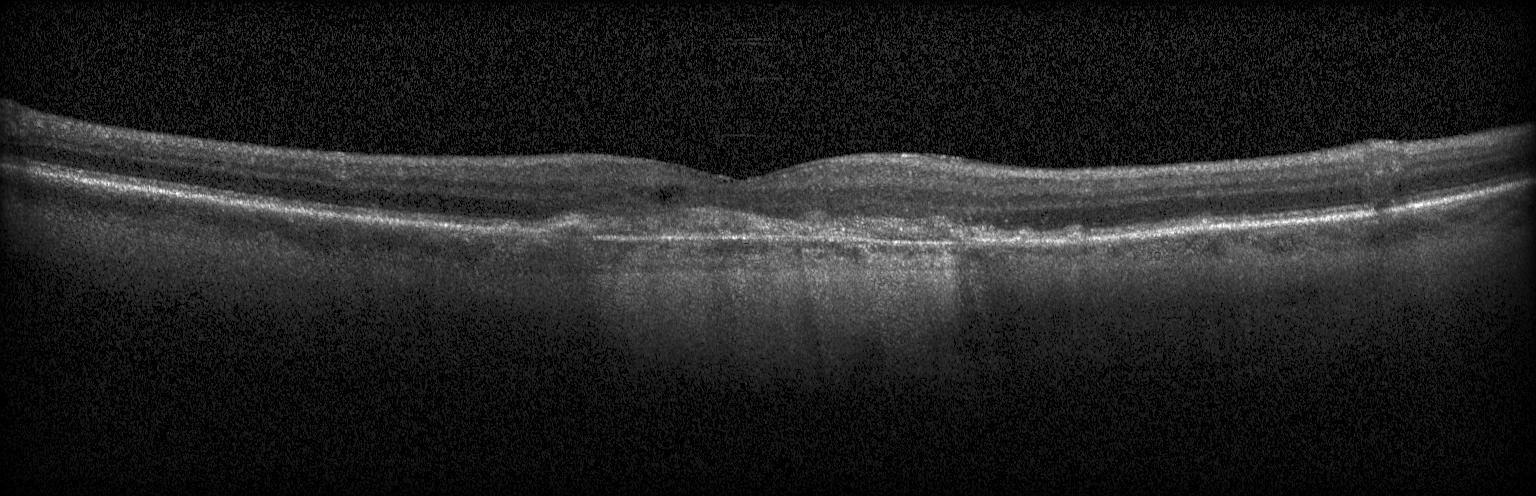 This B-scan demonstrates a choroidal neovascular membrane.